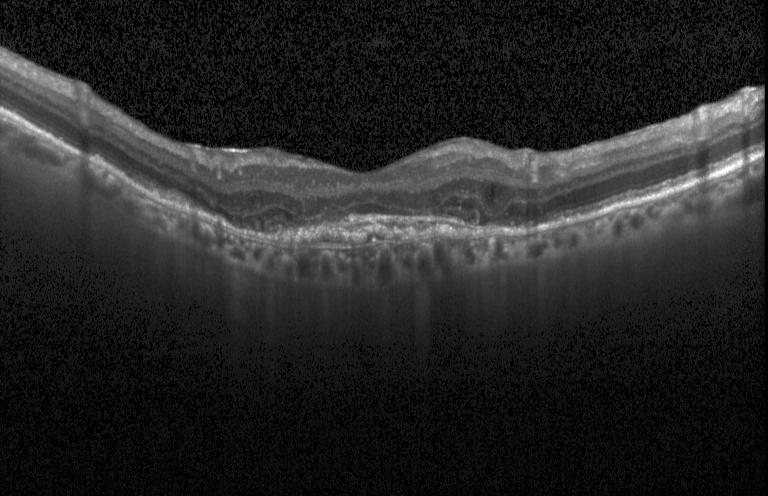 Diagnosis: choroidal neovascularization (CNV).